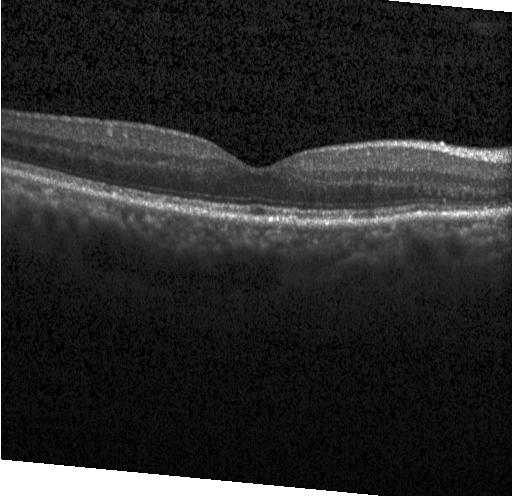

Instrument: Heidelberg Spectralis. Macular scan. Optical coherence tomography scan.
No choroidal neovascularization, no diabetic macular edema, and no drusen.